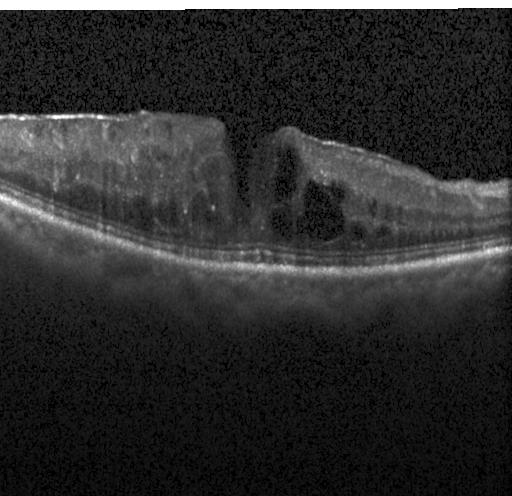

Diagnosis: diabetic macular edema.